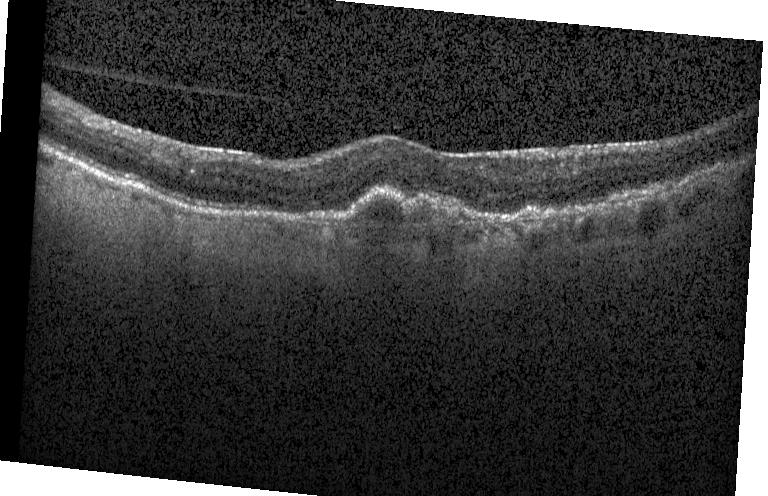

Retinal OCT B-scan.
Finding: a choroidal neovascular membrane.